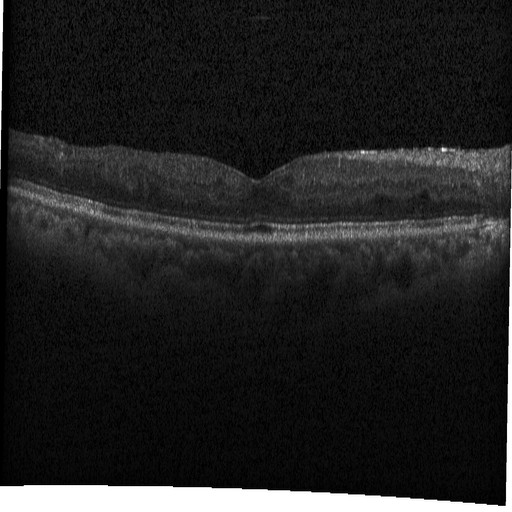

The scan shows diabetic macular edema.